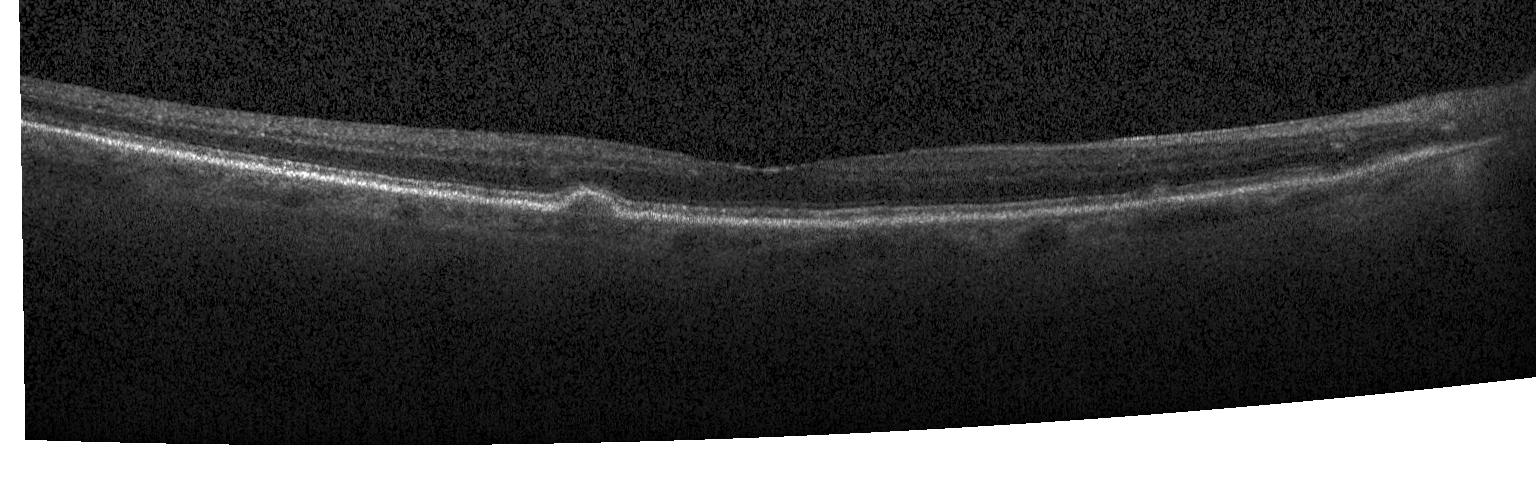

Retinal OCT cross-section showing sub-RPE drusenoid deposits.